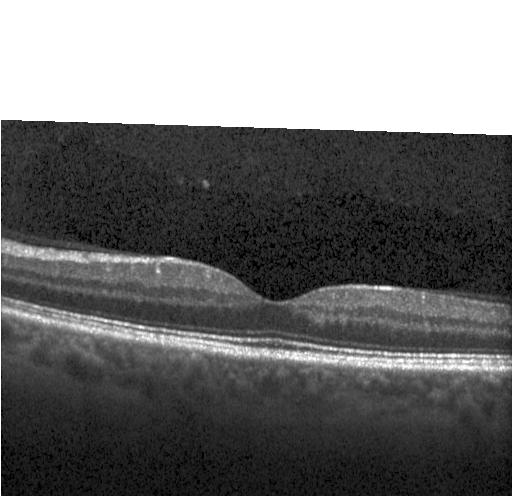

Retinal OCT B-scan
Impression: no evidence of CNV, DME, or drusen.